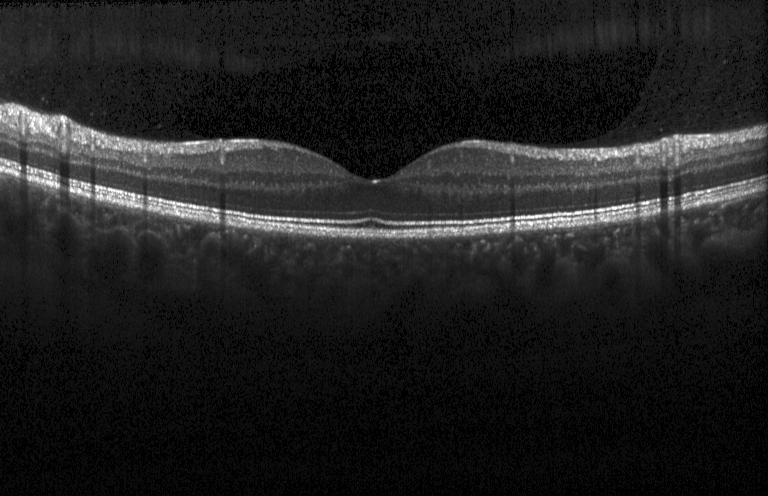

Acquired on a Heidelberg Spectralis, fovea-centered, SD-OCT, OCT B-scan.
Finding: neither choroidal neovascularization, diabetic macular edema, nor drusen.